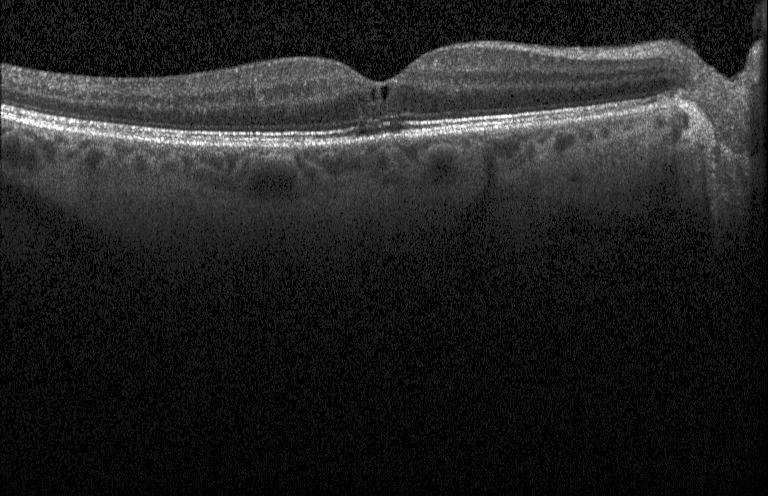 Spectral-domain OCT. Centered on the fovea. Retinal OCT B-scan. Heidelberg Spectralis OCT system.
This B-scan demonstrates diabetic macular edema.